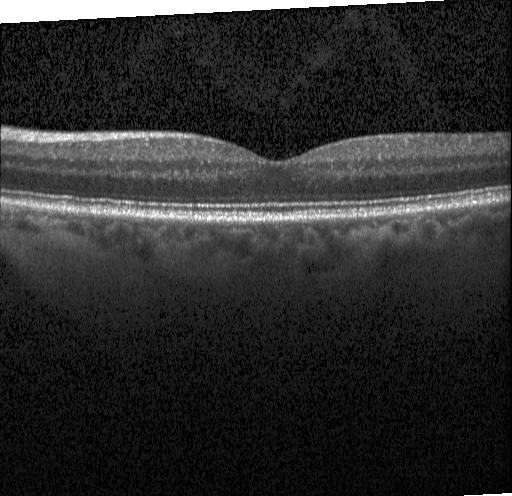 Neither choroidal neovascularization, diabetic macular edema, nor drusen.